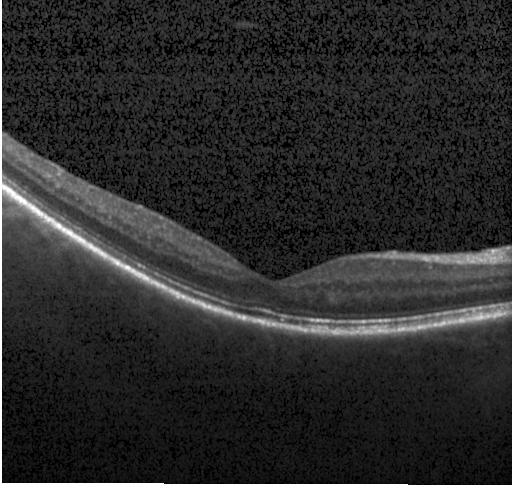
OCT B-scan, spectral-domain OCT, centered on the fovea, acquired on a Heidelberg Spectralis — Diagnosis: no choroidal neovascularization, no diabetic macular edema, and no drusen.